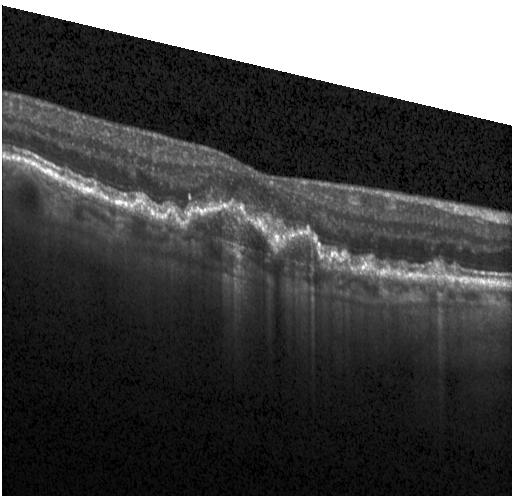 Impression: CNV.